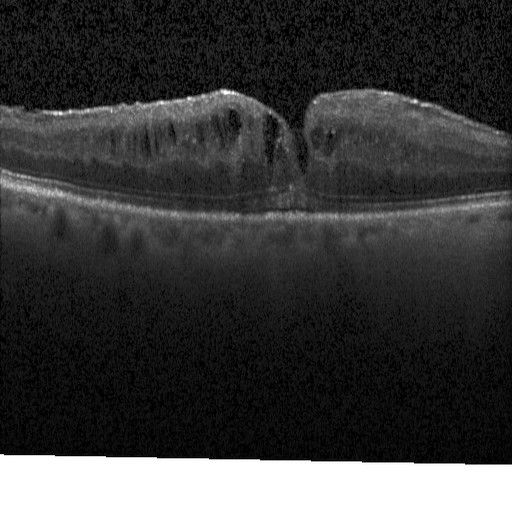 Diabetic macular edema.